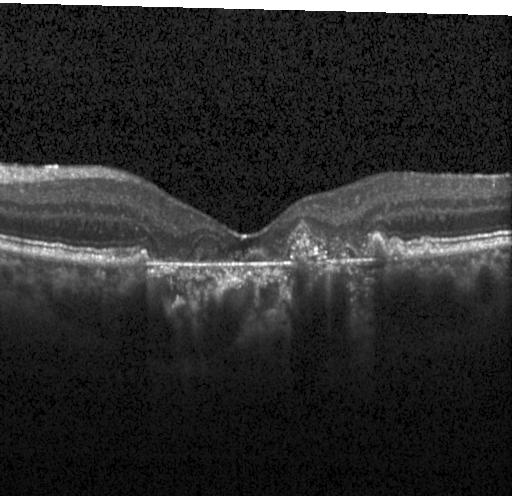

Fovea-centered · acquired on a Heidelberg Spectralis · OCT line scan.
Finding: a choroidal neovascular membrane.